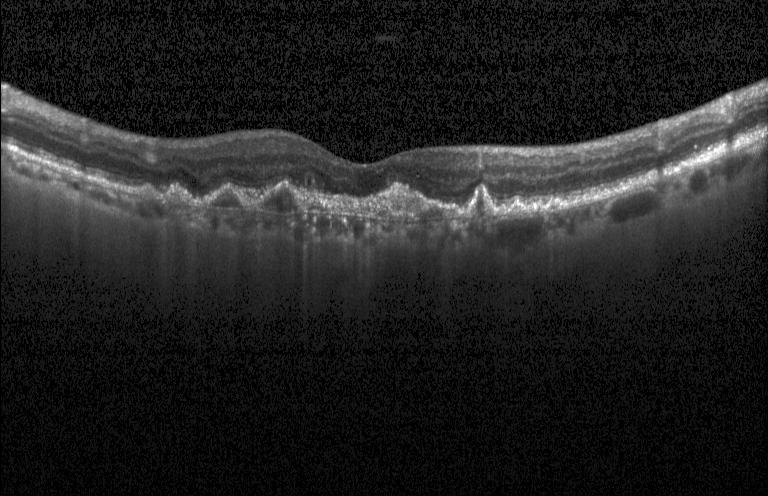 Assessment: CNV.